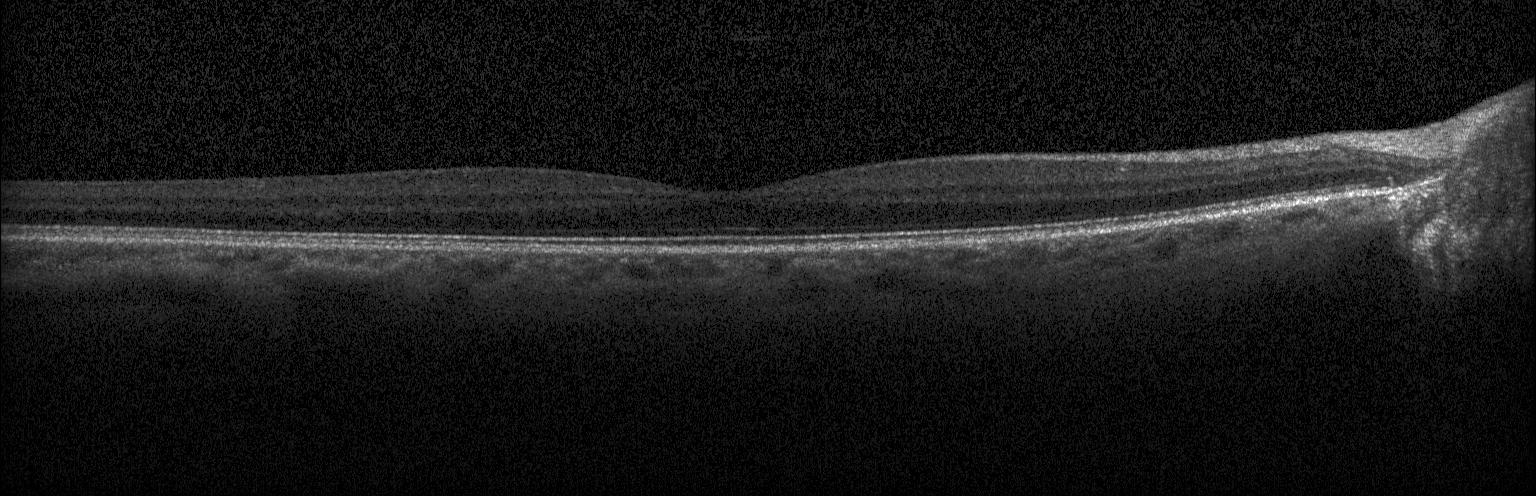

SD-OCT, optical coherence tomography B-scan, Heidelberg Spectralis
Impression: neither choroidal neovascularization, diabetic macular edema, nor drusen.